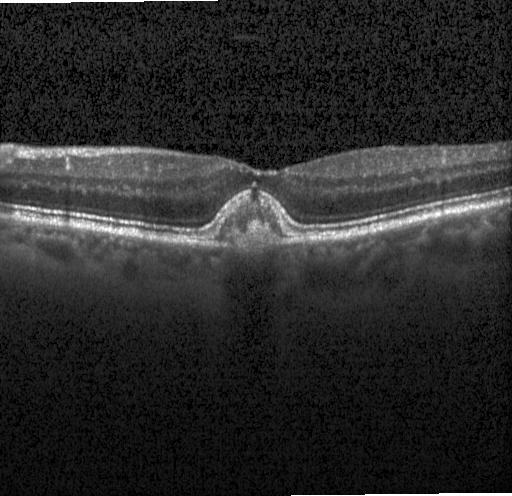 Optical coherence tomography B-scan, Heidelberg Spectralis OCT system, spectral-domain optical coherence tomography, through the macula — Finding: a choroidal neovascular membrane.